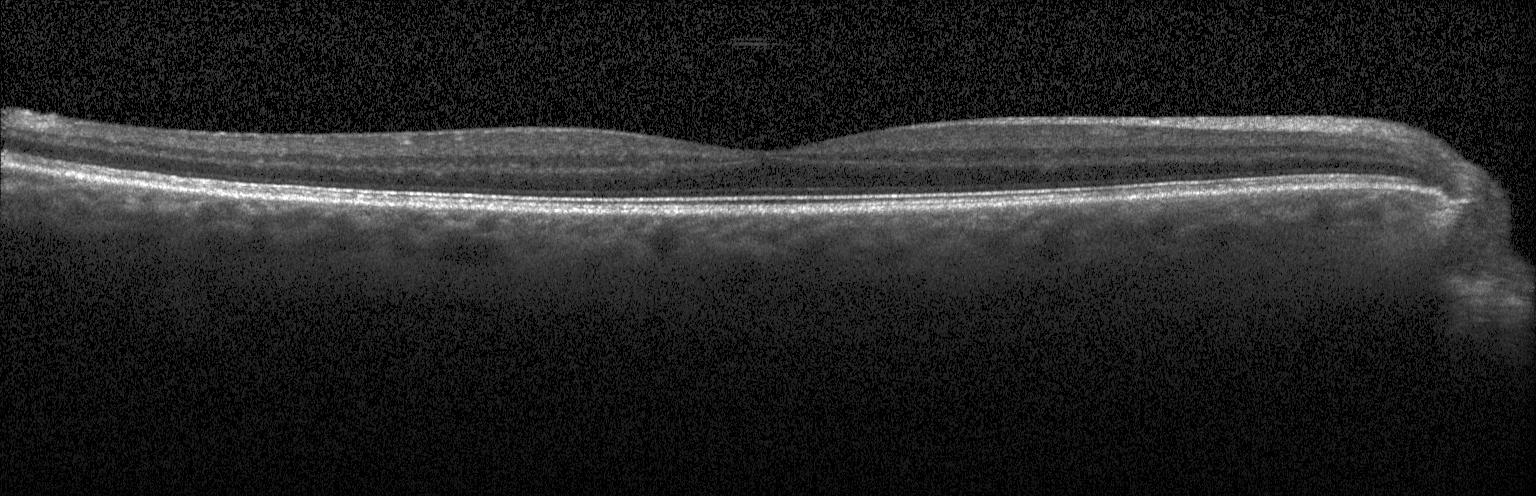

Acquired on a Heidelberg Spectralis. Retinal OCT B-scan. Through the macula. Finding: no CNV, DME, or drusen.